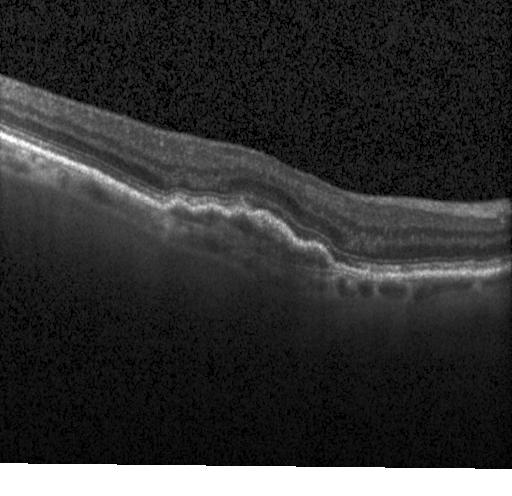 Assessment: a choroidal neovascular membrane.